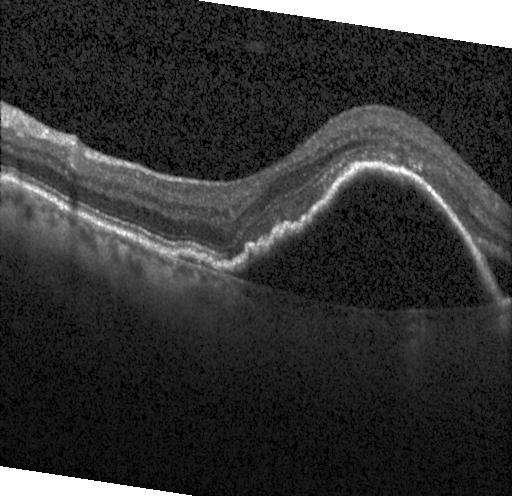 OCT B-scan; centered on the fovea; instrument: Heidelberg Spectralis; spectral-domain optical coherence tomography. This B-scan demonstrates choroidal neovascularization.